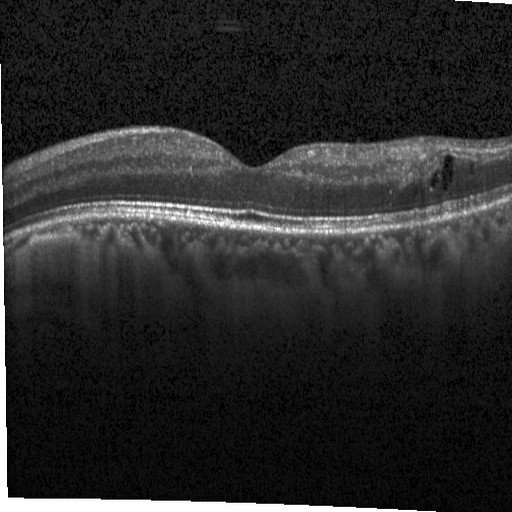 Retinal OCT cross-section showing diabetic macular edema (DME).